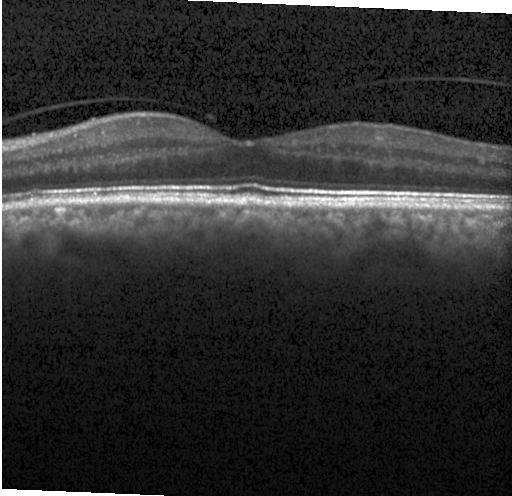

Retinal OCT B-scan; spectral-domain optical coherence tomography; centered on the fovea; acquired on a Heidelberg Spectralis — The scan shows no evidence of CNV, DME, or drusen.